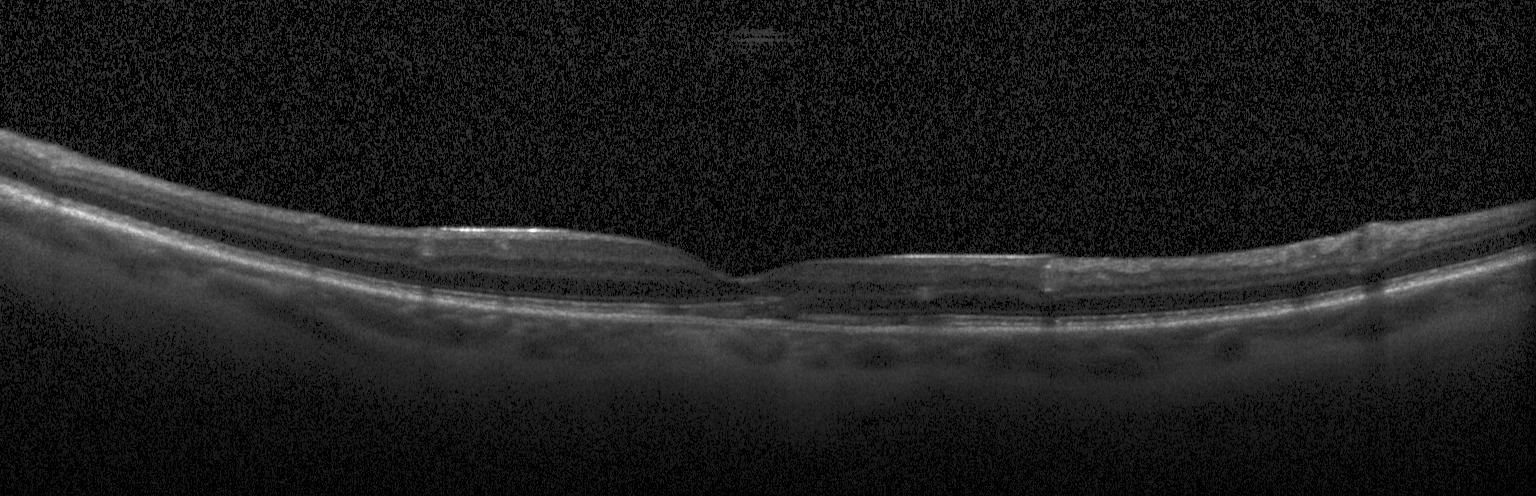
OCT line scan. This B-scan demonstrates a choroidal neovascular membrane.